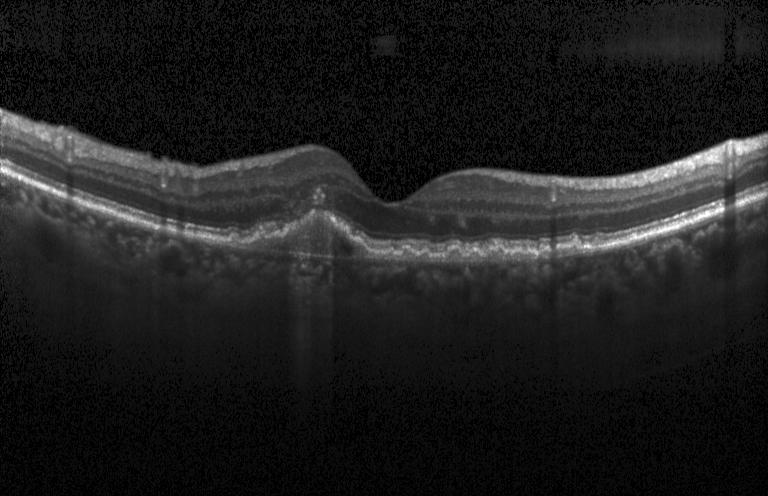

Retinal OCT cross-section, fovea-centered.
OCT finding: a choroidal neovascular membrane.